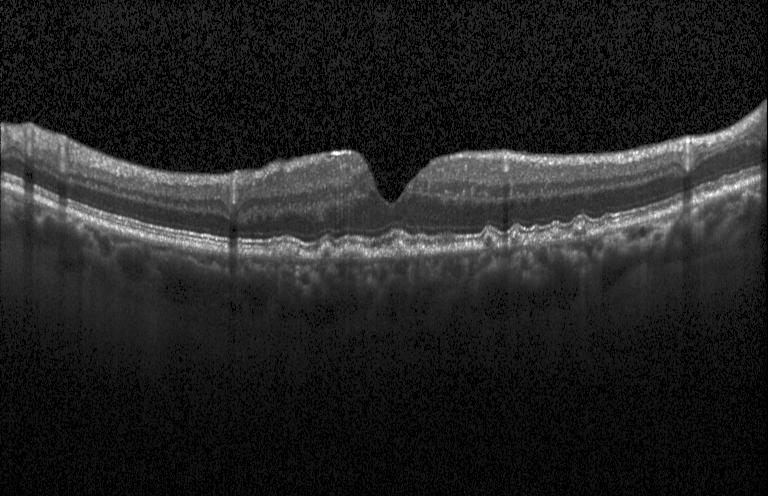

Acquired on a Heidelberg Spectralis; macular scan; optical coherence tomography B-scan — Drusen.